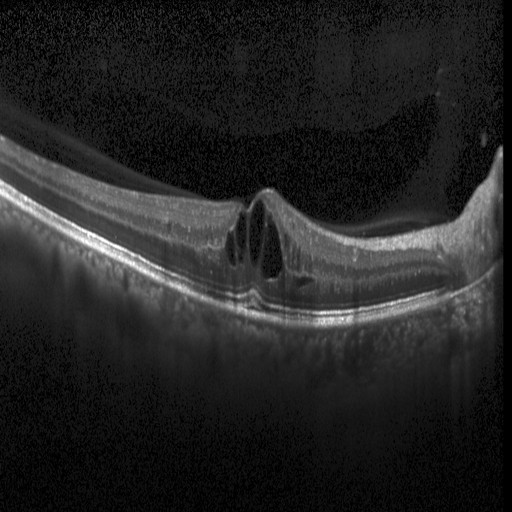 Macular OCT demonstrating diabetic macular edema (DME).